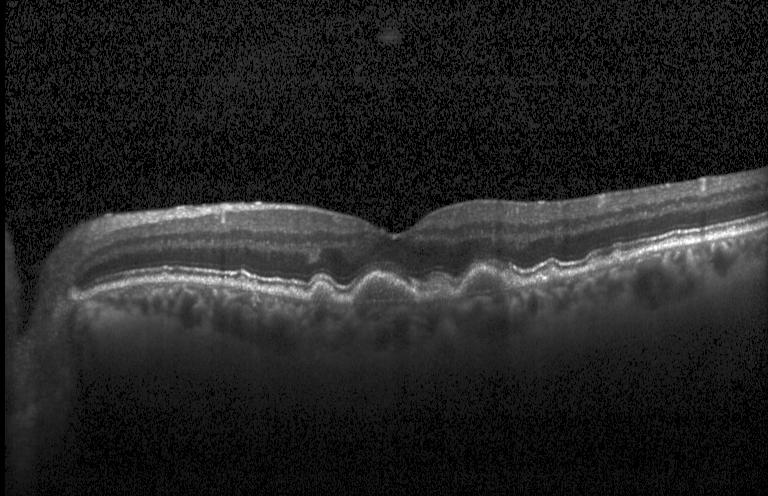

Spectral-domain OCT. Horizontal scan through the fovea. Optical coherence tomography scan.
Impression: multiple drusen.